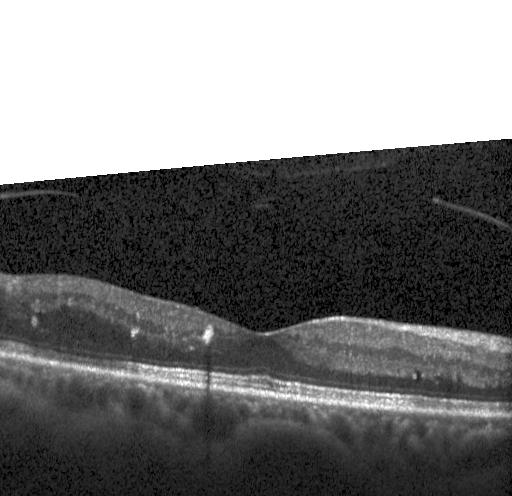 Optical coherence tomography B-scan · fovea-centered
Diagnosis: diabetic macular edema (DME).